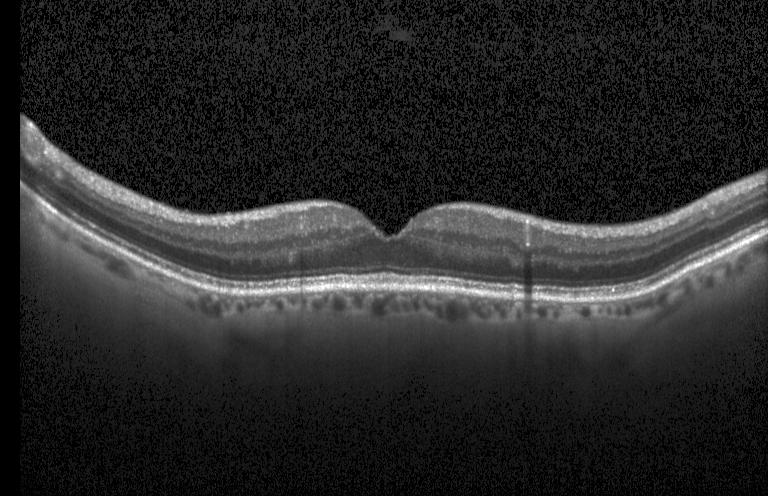
Spectral-domain OCT · acquired on a Heidelberg Spectralis · OCT B-scan · centered on the fovea — This B-scan demonstrates no CNV, no DME, and no drusen.